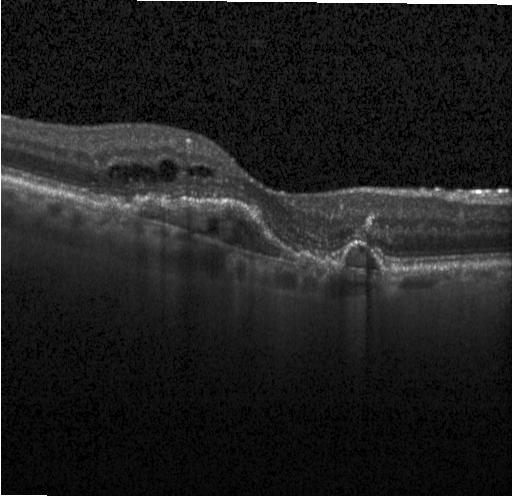

Centered on the fovea; spectral-domain OCT; retinal OCT cross-section. Diagnosis: CNV.